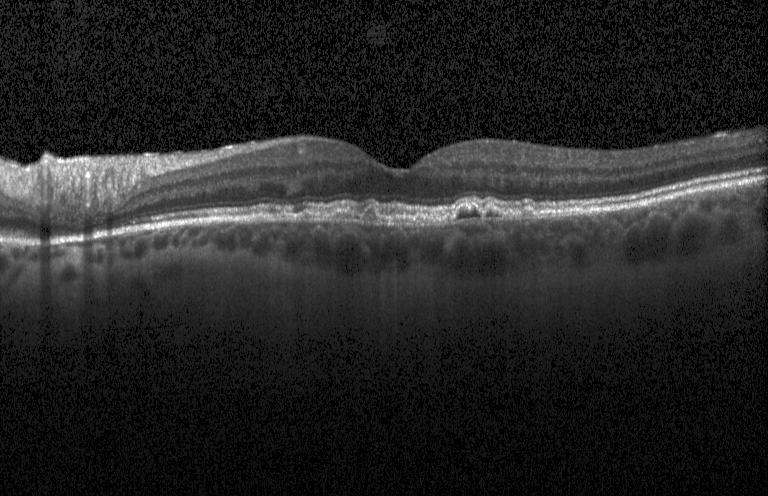 Retinal OCT cross-section; macular scan.
Assessment: multiple drusen.